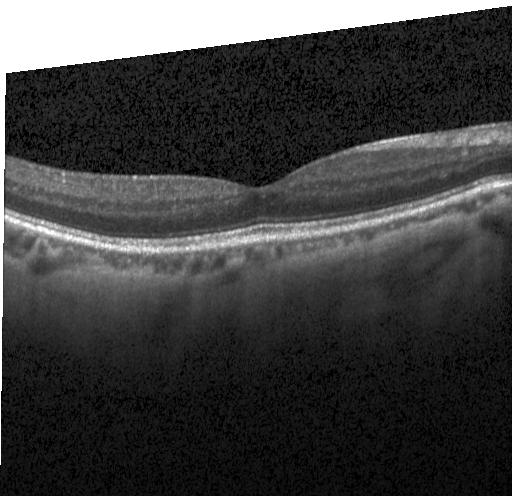
Horizontal scan through the fovea, retinal OCT B-scan
No choroidal neovascularization, diabetic macular edema, or drusen.